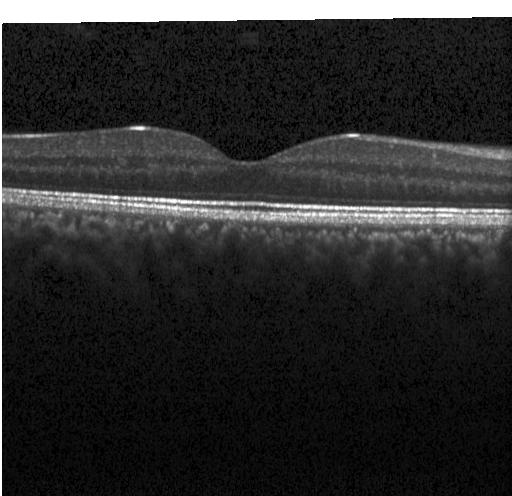 Retinal OCT cross-section. Diagnosis: no evidence of choroidal neovascularization, diabetic macular edema, or drusen.